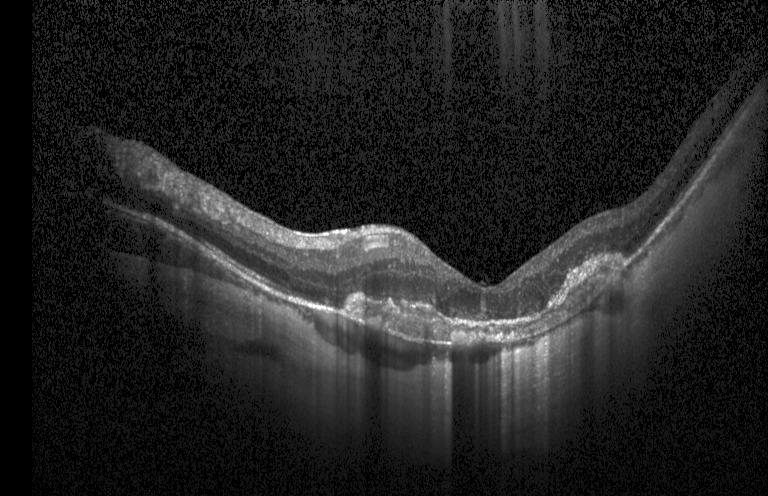 OCT B-scan showing CNV.